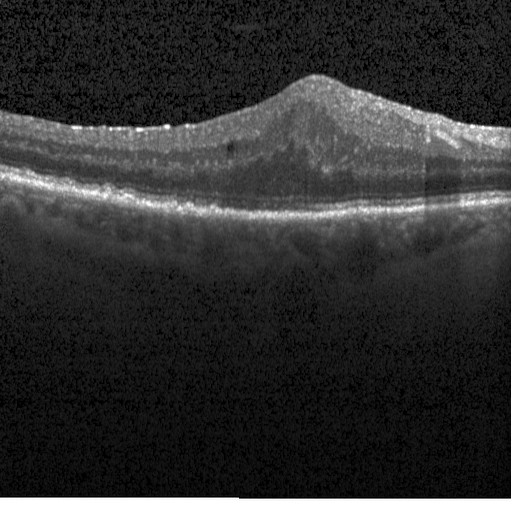
Optical coherence tomography scan. Horizontal scan through the fovea. Impression: diabetic macular edema.